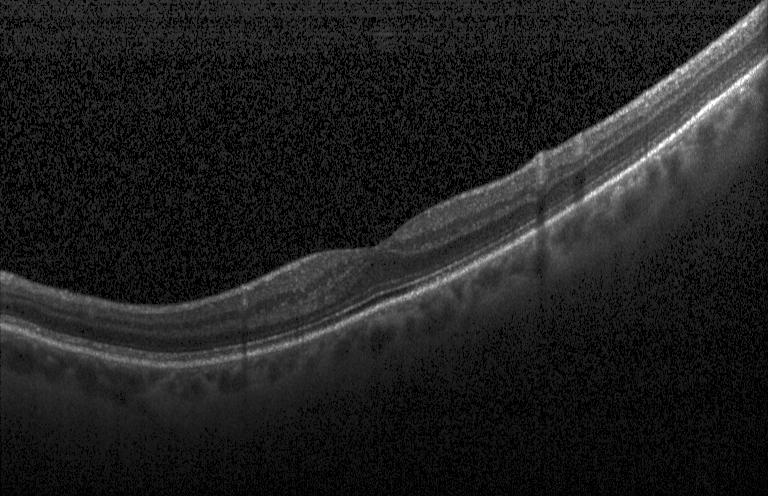

OCT B-scan showing no CNV, DME, or drusen.